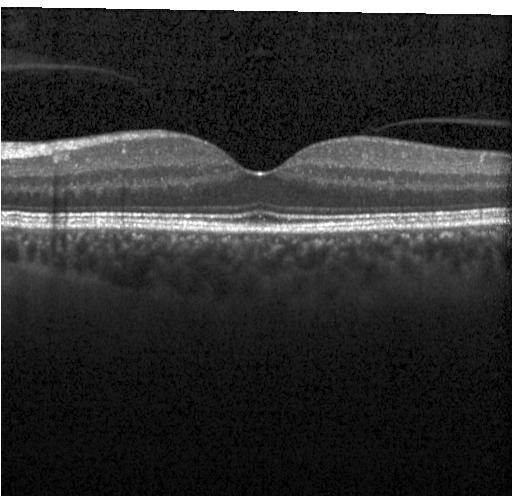 Diagnosis: no choroidal neovascularization, no diabetic macular edema, and no drusen.